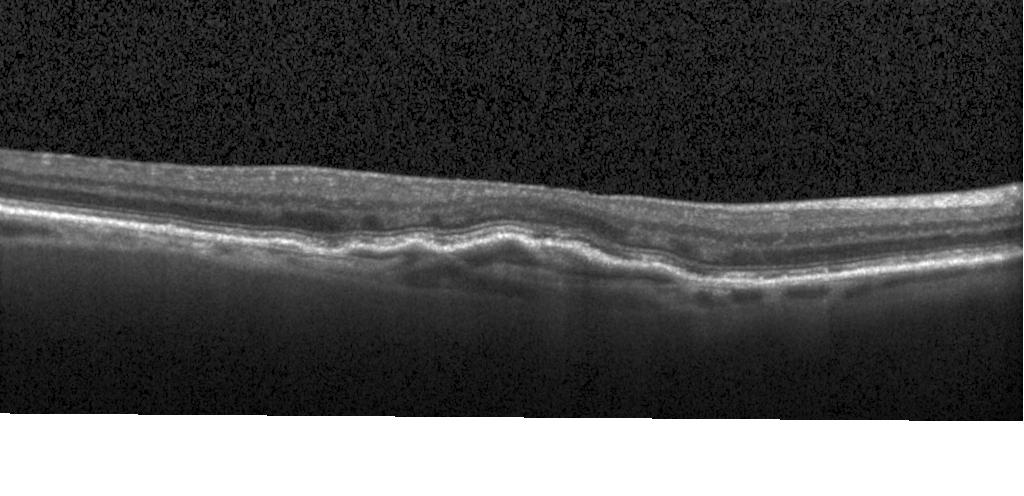

The scan shows a choroidal neovascular membrane.